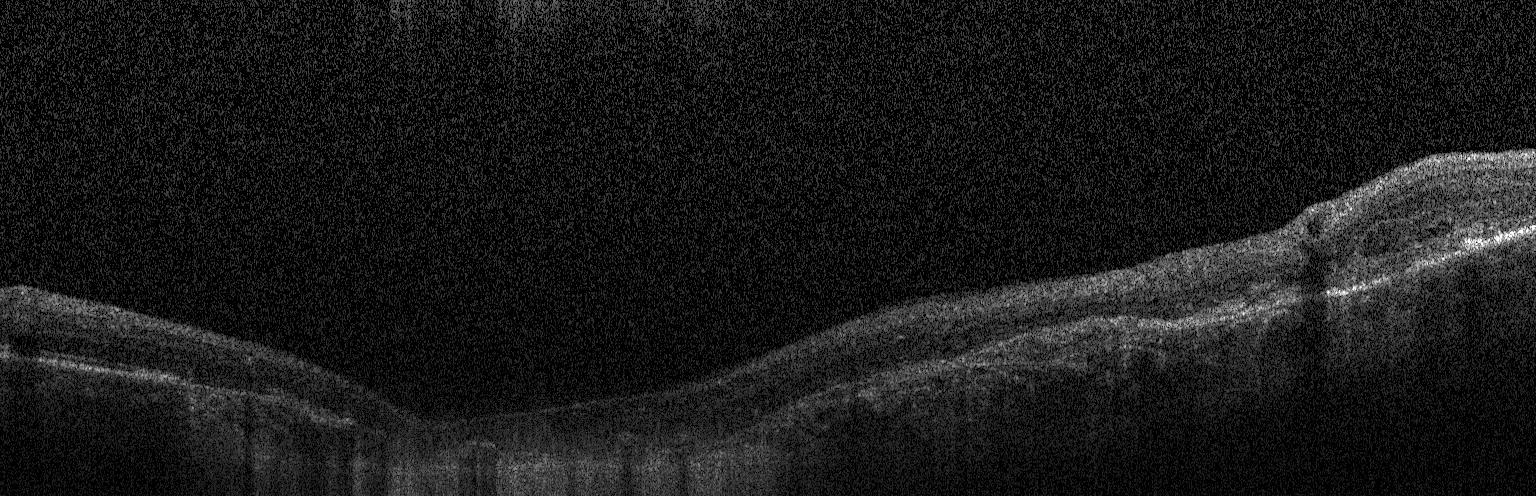

Spectral-domain OCT; optical coherence tomography scan — Dx: a choroidal neovascular membrane.